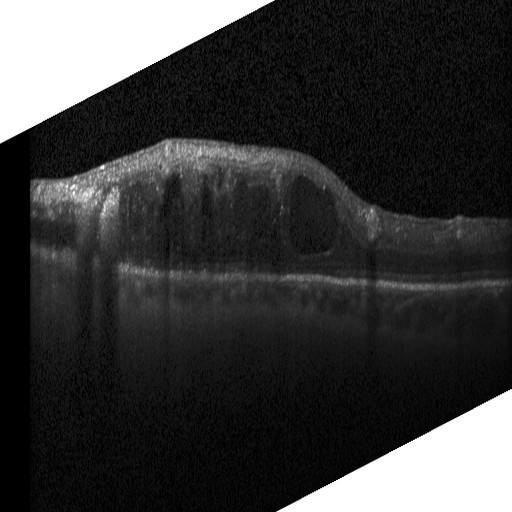

Finding: diabetic macular edema.